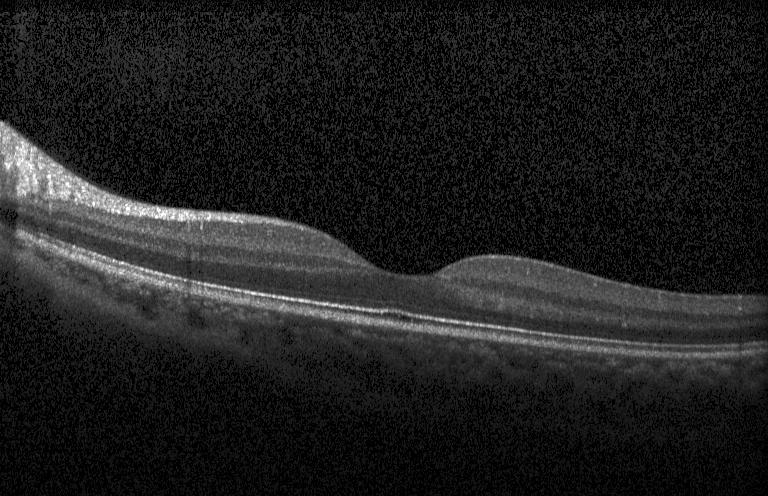
Dx: no choroidal neovascularization, diabetic macular edema, or drusen.